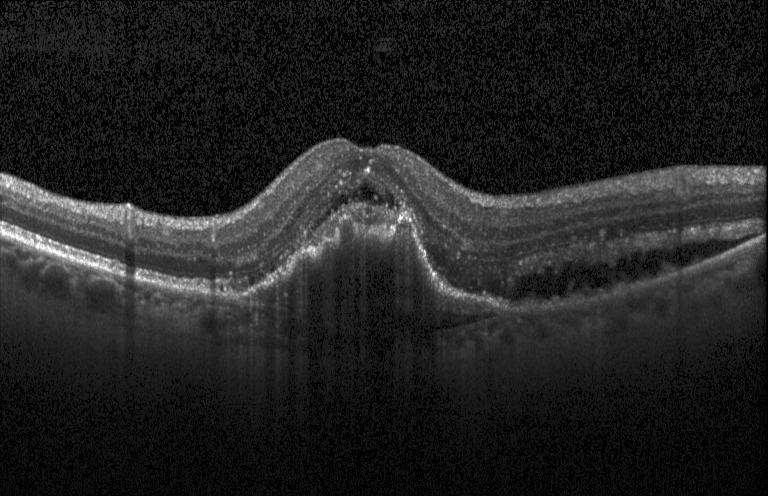 Retinal OCT cross-section. Diagnosis: a choroidal neovascular membrane.